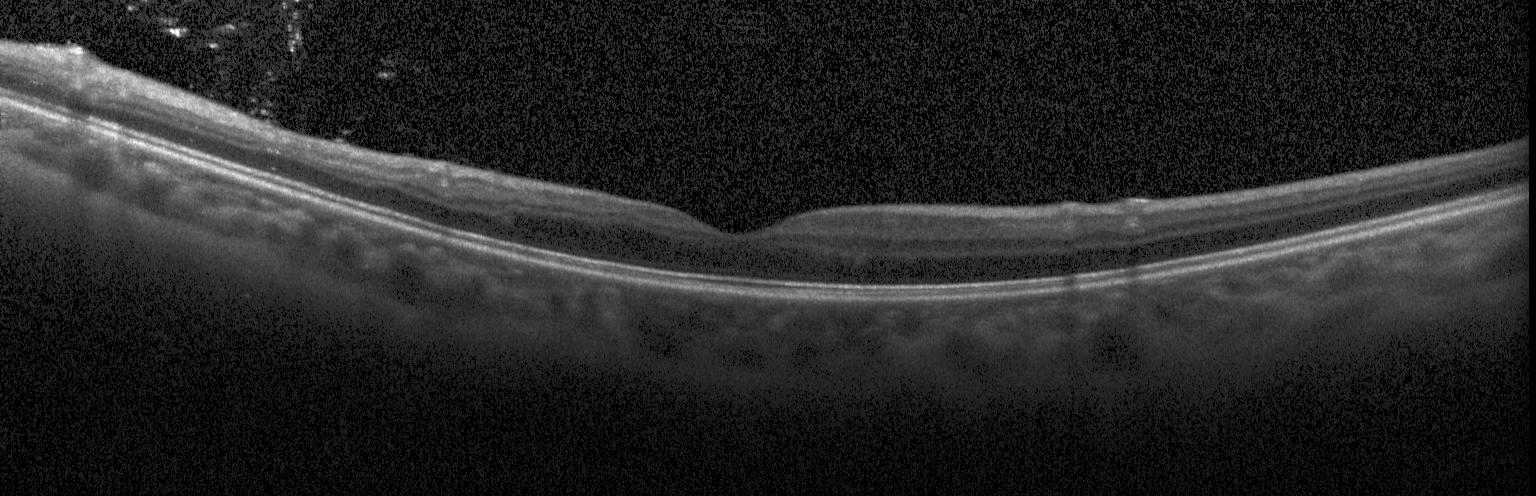

Diagnosis: no evidence of CNV, DME, or drusen.